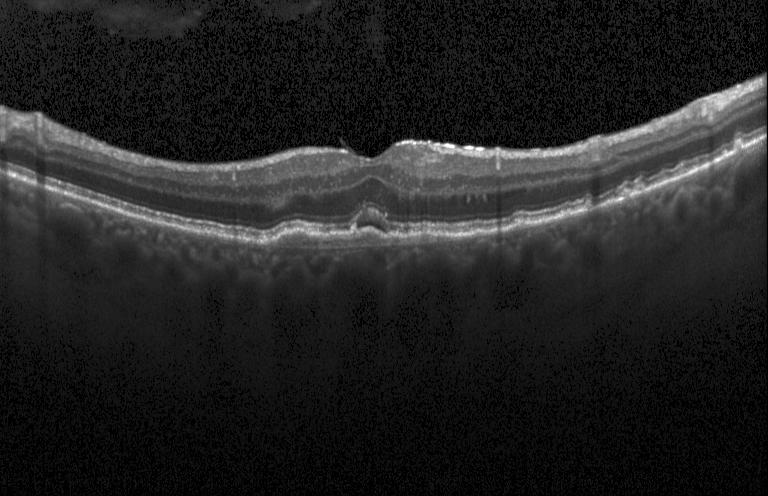 A choroidal neovascular membrane.